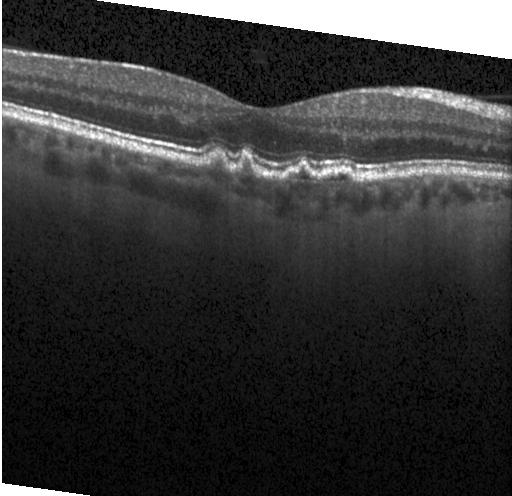
Macular OCT: sub-RPE drusenoid deposits.